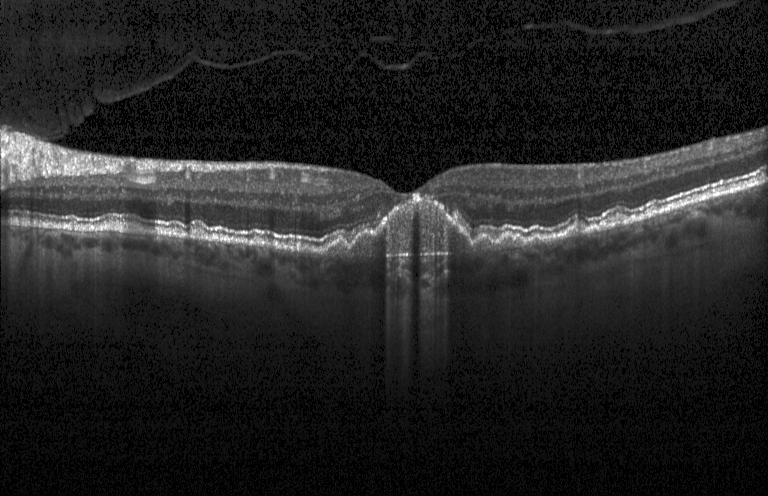
Retinal OCT B-scan
Macular OCT: CNV.